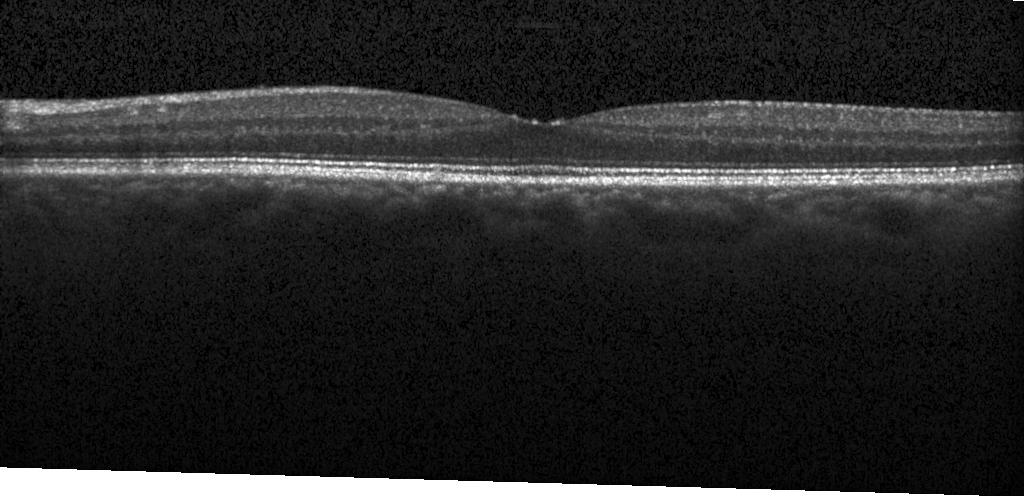

Retinal OCT B-scan, centered on the fovea. Diagnosis: no evidence of choroidal neovascularization, diabetic macular edema, or drusen.